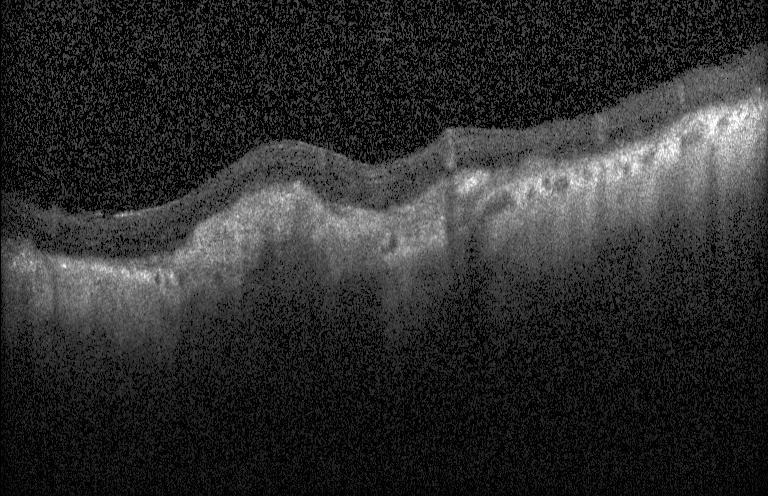
SD-OCT. Heidelberg Spectralis. Retinal OCT cross-section. Macular scan. The scan shows a choroidal neovascular membrane.